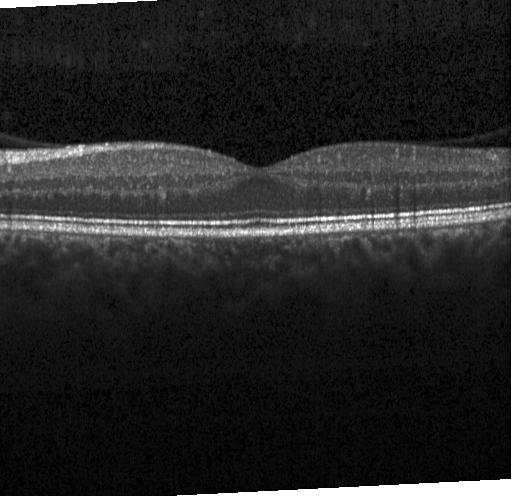
Finding: neither choroidal neovascularization, diabetic macular edema, nor drusen.